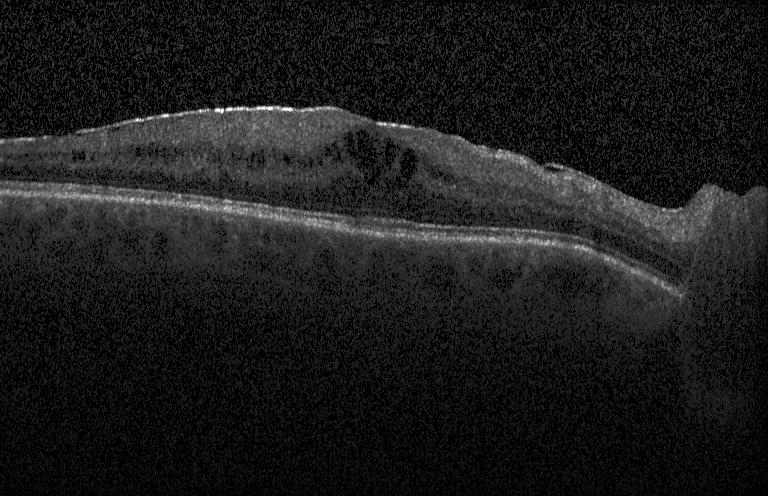
Retinal OCT cross-section.
This B-scan demonstrates diabetic macular edema.